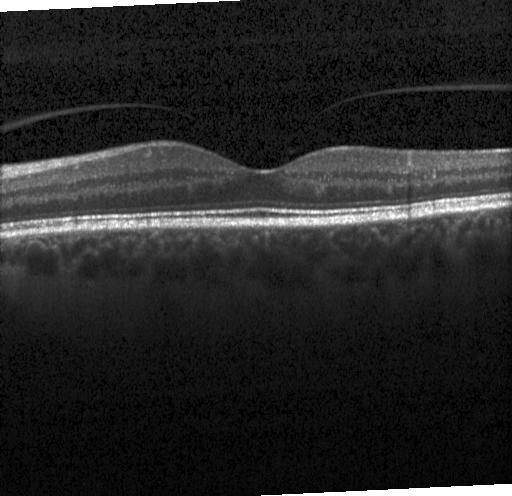

Retinal OCT cross-section · instrument: Heidelberg Spectralis. Impression: no choroidal neovascularization, diabetic macular edema, or drusen.